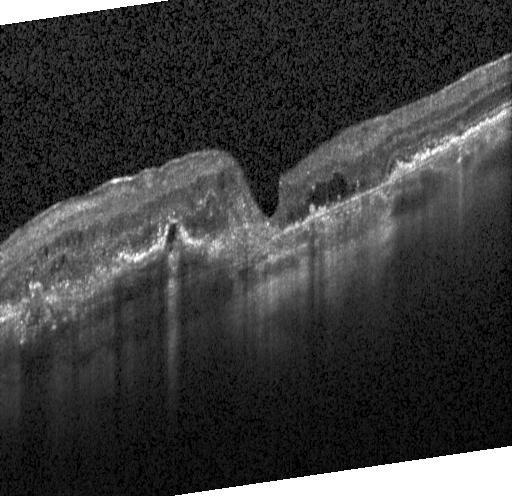 OCT line scan. Instrument: Heidelberg Spectralis. Fovea-centered. Spectral-domain optical coherence tomography.
The scan shows choroidal neovascularization.